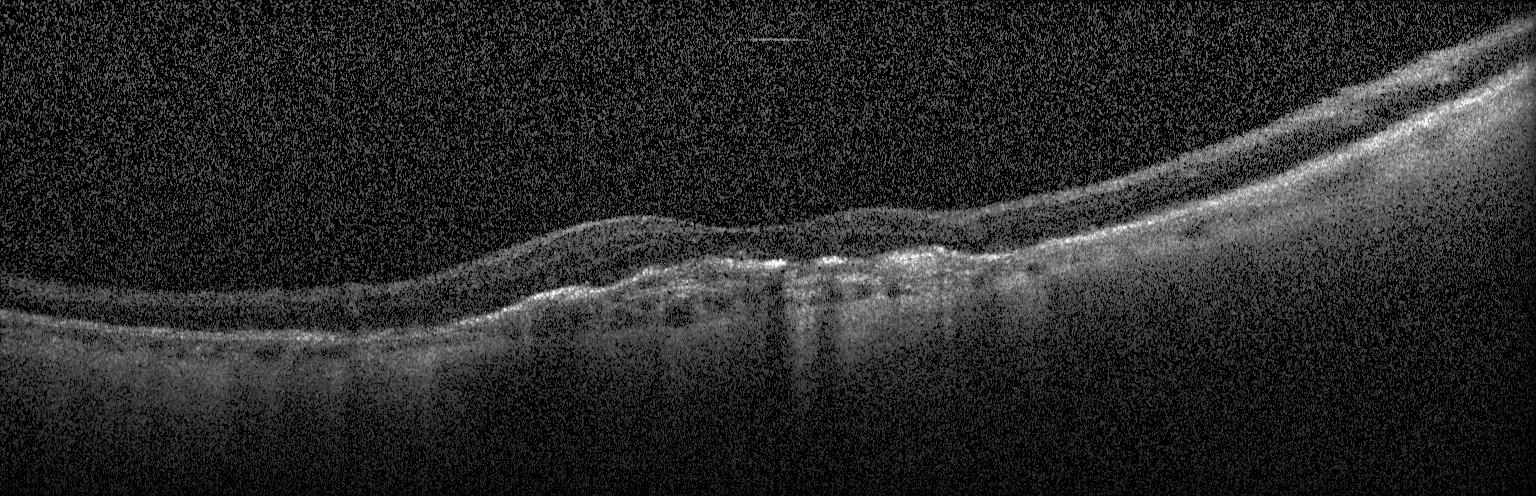 Spectral-domain optical coherence tomography · horizontal scan through the fovea · OCT line scan.
Diagnosis: choroidal neovascularization (CNV).